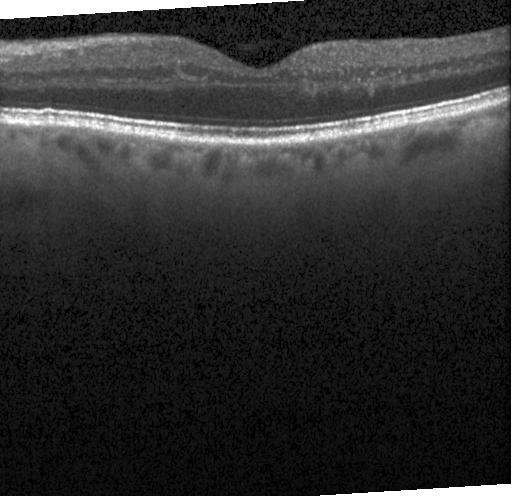
Finding: neither CNV, DME, nor drusen.